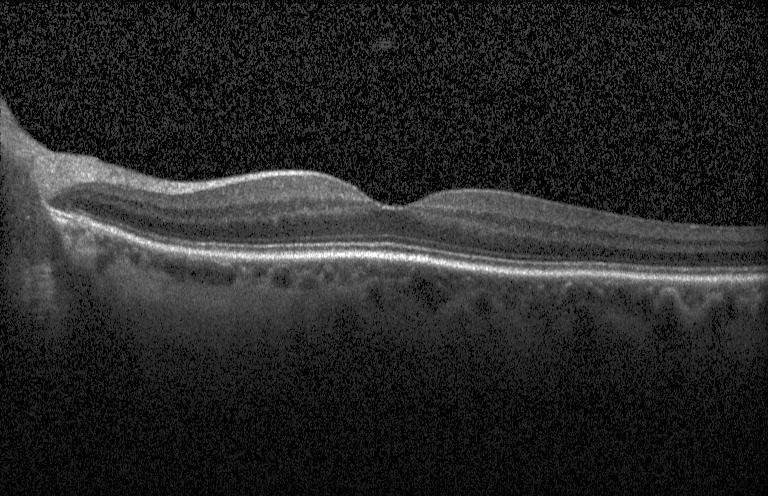

Finding: no choroidal neovascularization, diabetic macular edema, or drusen.